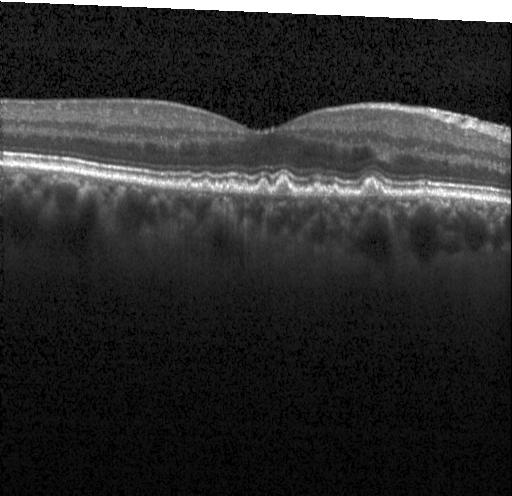
Acquired on a Heidelberg Spectralis, spectral-domain optical coherence tomography, OCT B-scan, fovea-centered. Impression: drusen.